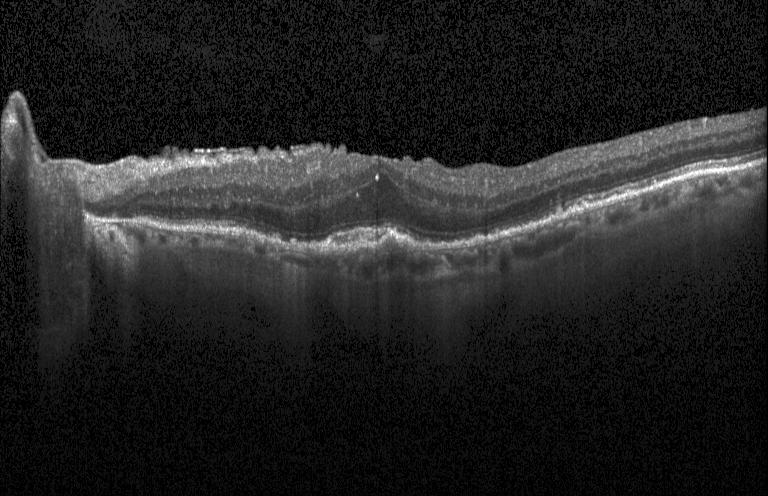 Retinal OCT B-scan · spectral-domain optical coherence tomography · Heidelberg Spectralis
Diagnosis: a choroidal neovascular membrane.